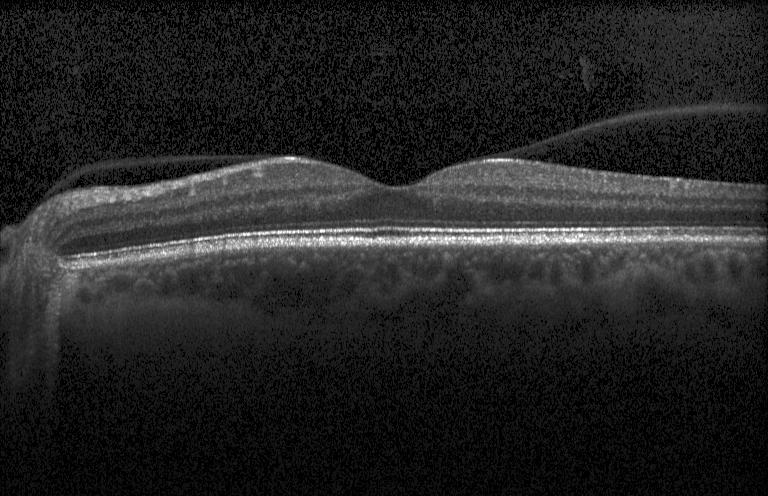

Dx: no CNV, DME, or drusen.